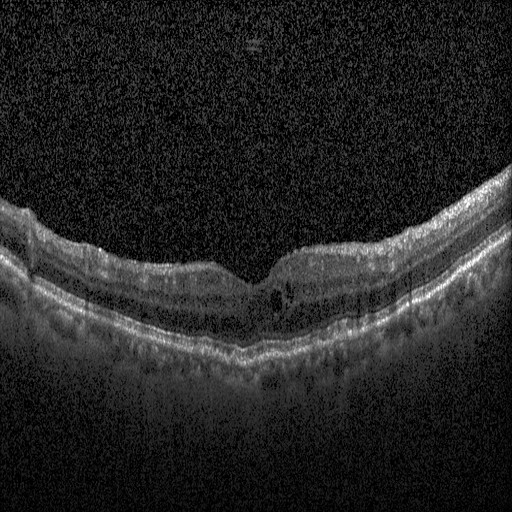
Instrument: Heidelberg Spectralis · retinal OCT cross-section
Finding: diabetic macular edema (DME).